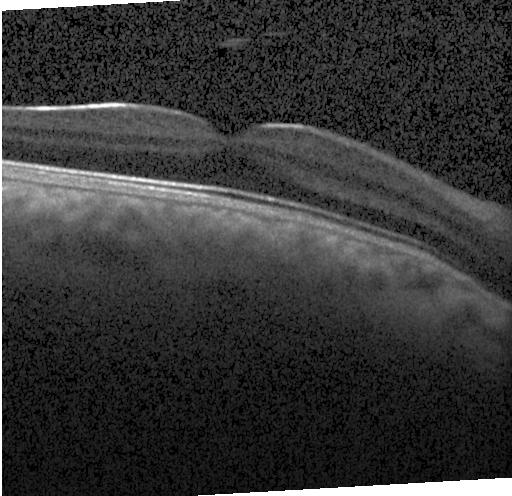

Impression: no choroidal neovascularization, diabetic macular edema, or drusen.